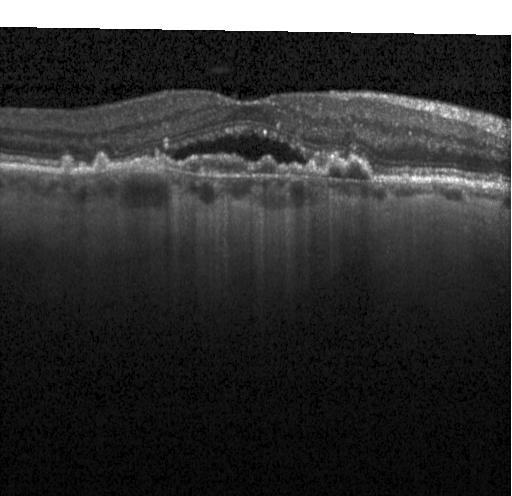

OCT scan showing a choroidal neovascular membrane.